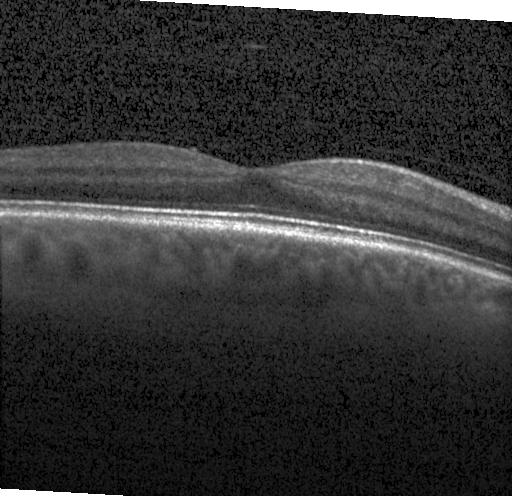

Heidelberg Spectralis · spectral-domain optical coherence tomography · retinal OCT cross-section · macular scan. No choroidal neovascularization, no diabetic macular edema, and no drusen.